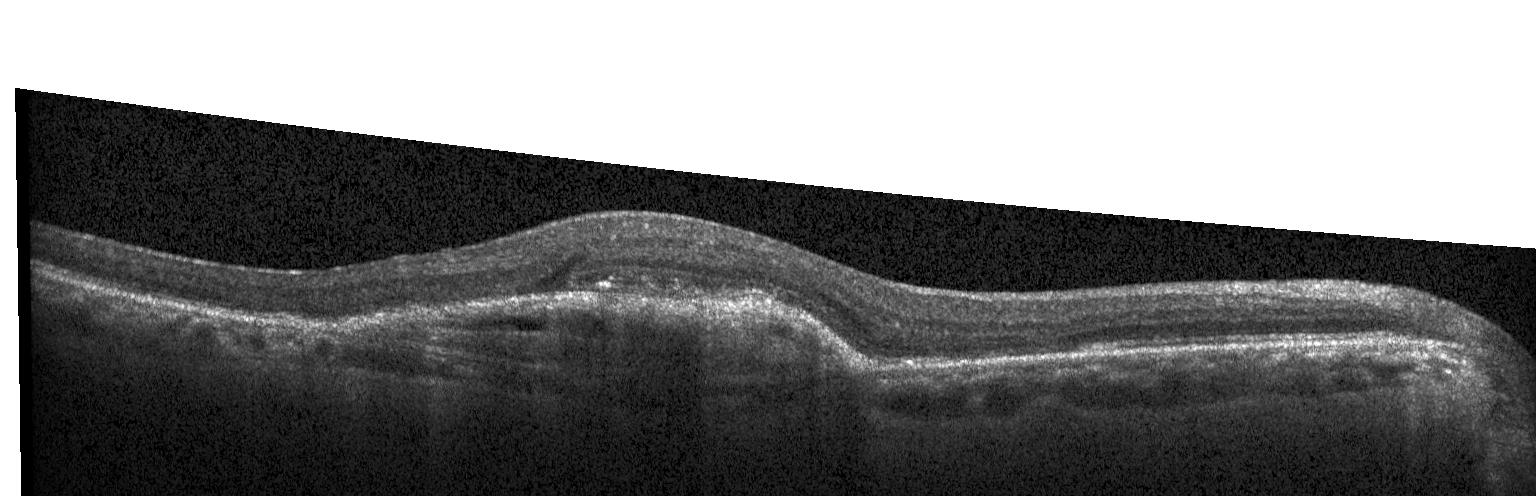
Diagnosis: a choroidal neovascular membrane.